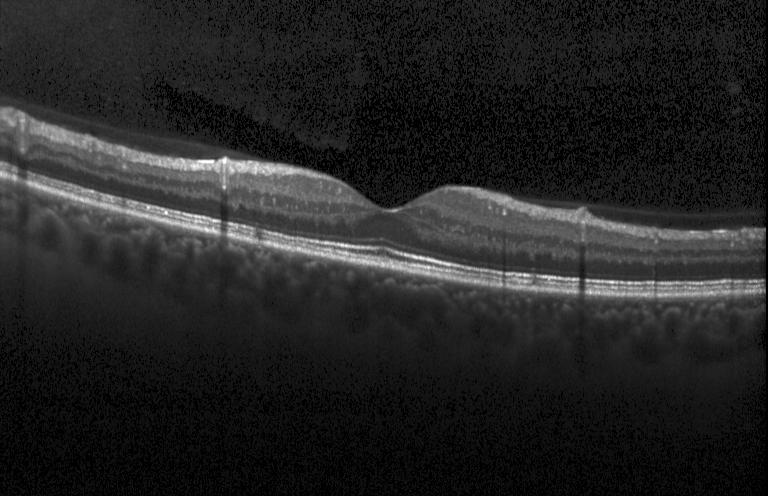

Diagnosis: neither choroidal neovascularization, diabetic macular edema, nor drusen.